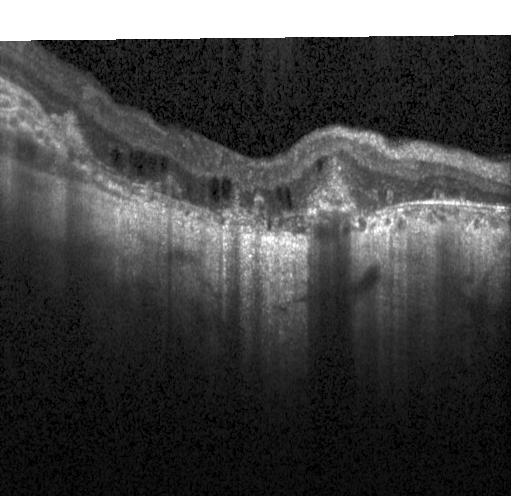
Spectral-domain OCT · centered on the fovea · Heidelberg Spectralis · optical coherence tomography B-scan
Assessment: choroidal neovascularization (CNV).